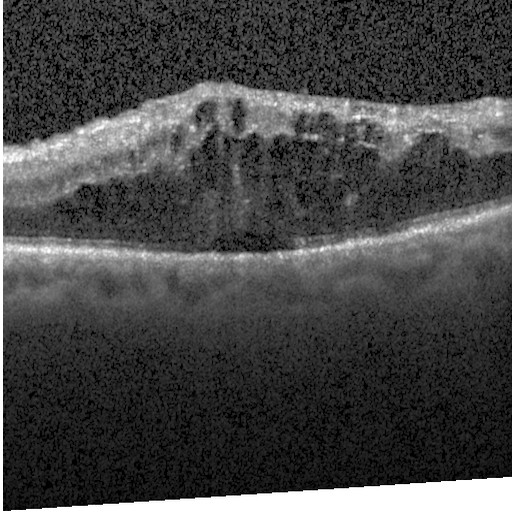

Retinal OCT B-scan; acquired on a Heidelberg Spectralis. Impression: diabetic macular edema.